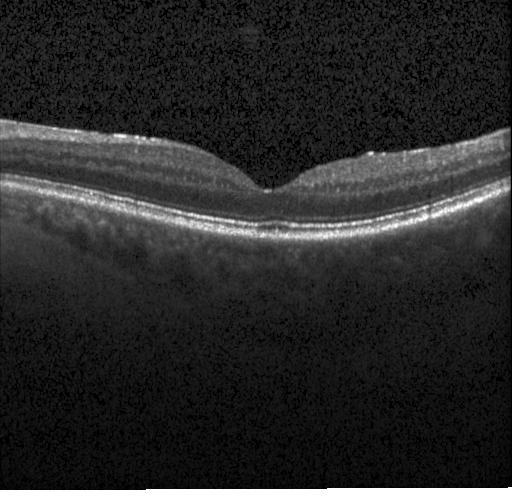

OCT line scan. Finding: no CNV, no DME, and no drusen.